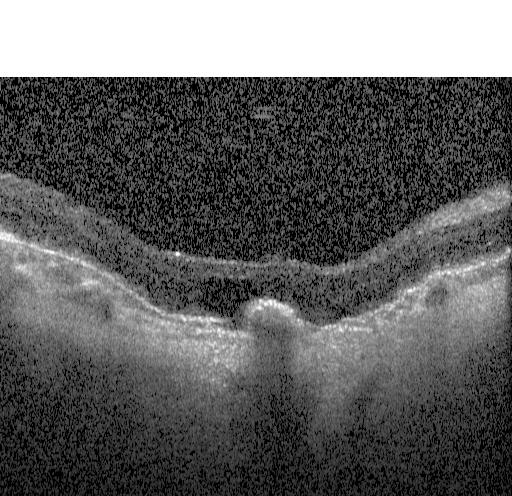
Heidelberg Spectralis OCT system; optical coherence tomography scan; spectral-domain optical coherence tomography
Diagnosis: choroidal neovascularization (CNV).